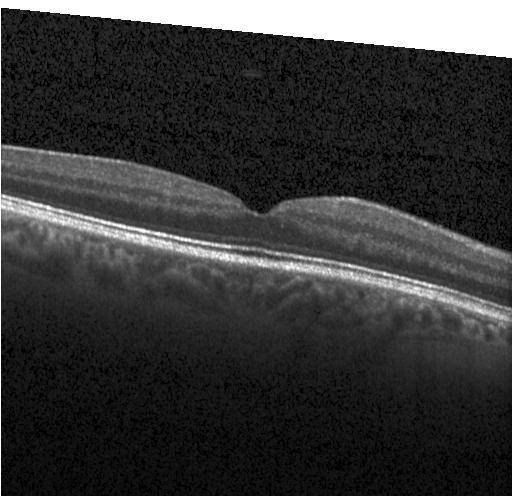

OCT line scan; spectral-domain optical coherence tomography; through the macula — Finding: no evidence of choroidal neovascularization, diabetic macular edema, or drusen.